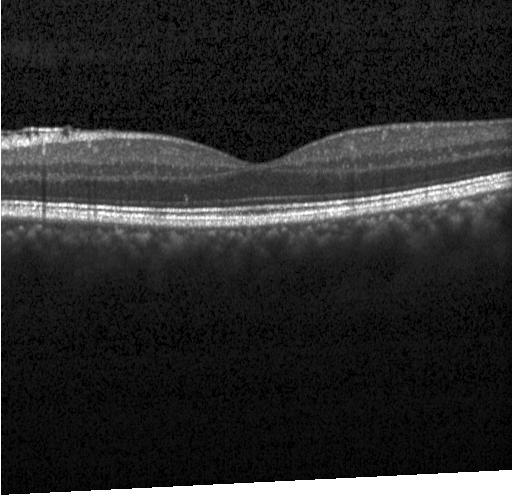

OCT finding: no choroidal neovascularization, diabetic macular edema, or drusen.